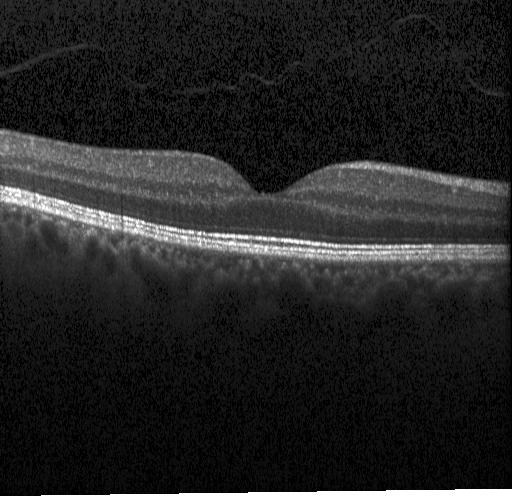

OCT scan showing neither choroidal neovascularization, diabetic macular edema, nor drusen.